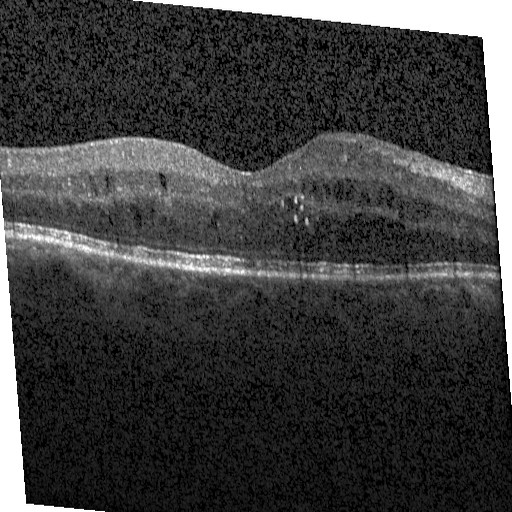
Macular scan · retinal OCT B-scan · spectral-domain optical coherence tomography. Diagnosis: diabetic macular edema.